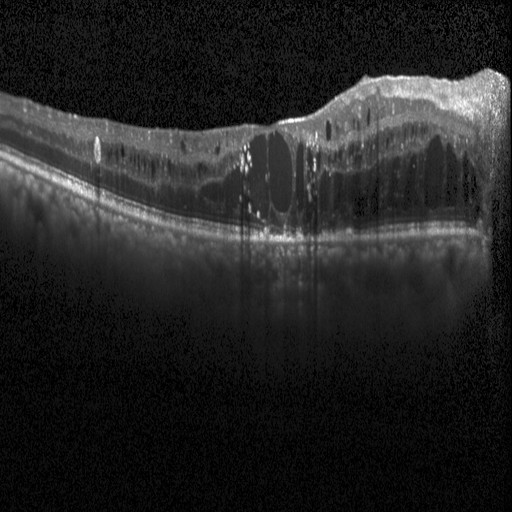 SD-OCT, macular scan, optical coherence tomography B-scan
Impression: diabetic macular edema (DME).